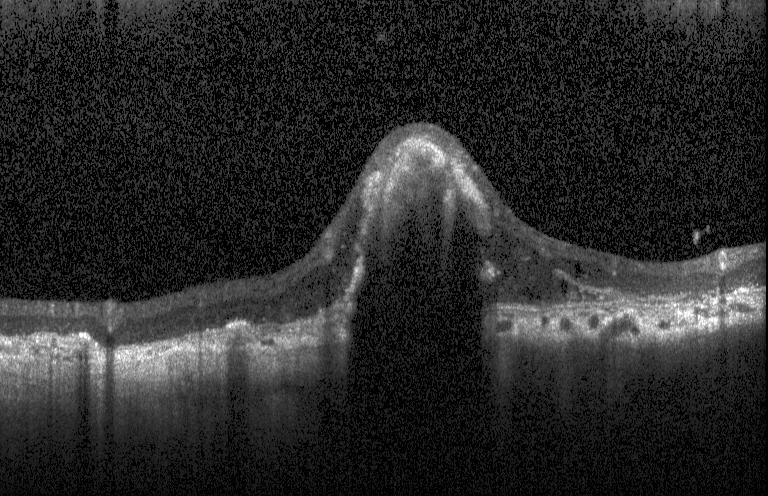 OCT B-scan. Macular OCT: a choroidal neovascular membrane.